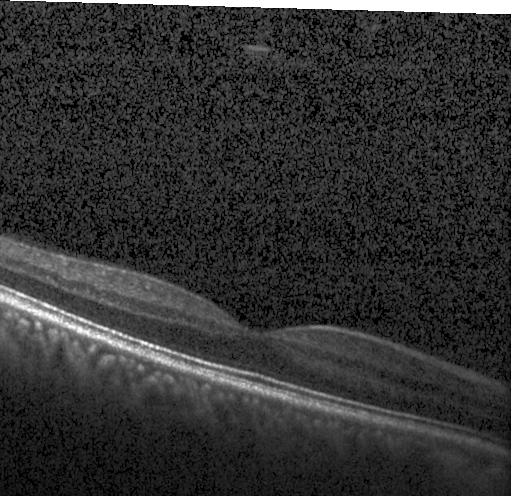
Optical coherence tomography scan · centered on the fovea.
This B-scan demonstrates no choroidal neovascularization, diabetic macular edema, or drusen.